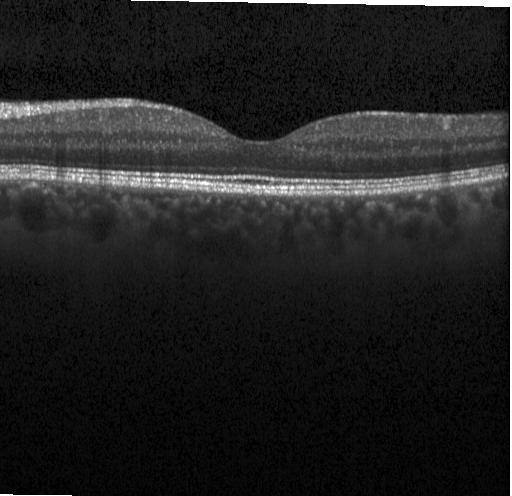

Optical coherence tomography scan, instrument: Heidelberg Spectralis.
Diagnosis: no CNV, no DME, and no drusen.